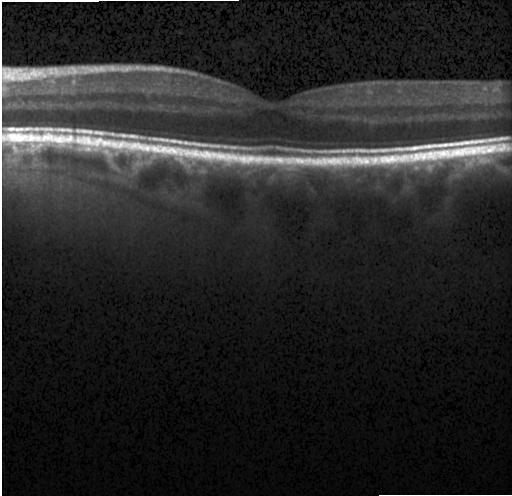
Macular OCT: neither choroidal neovascularization, diabetic macular edema, nor drusen.